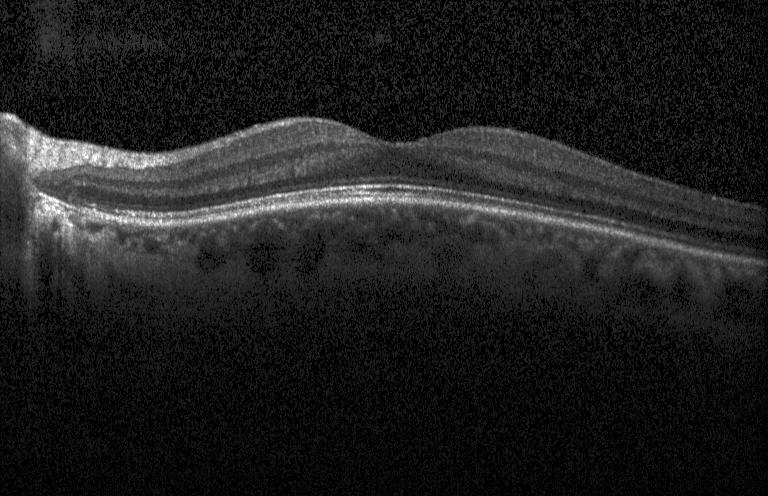 Diagnosis: no choroidal neovascularization, no diabetic macular edema, and no drusen.